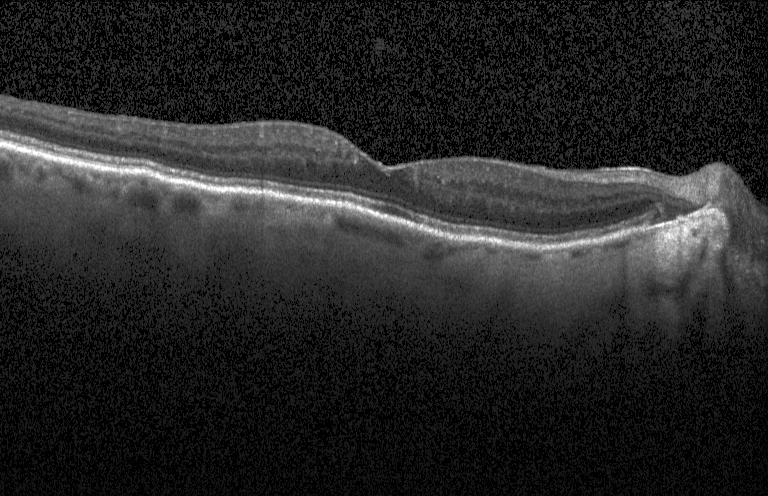
Macular OCT demonstrating no evidence of choroidal neovascularization, diabetic macular edema, or drusen.